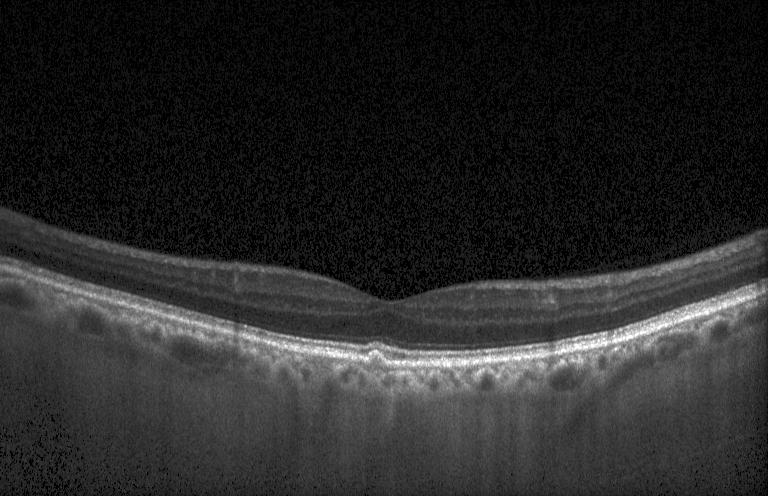
Spectral-domain OCT B-scan: sub-RPE drusenoid deposits.